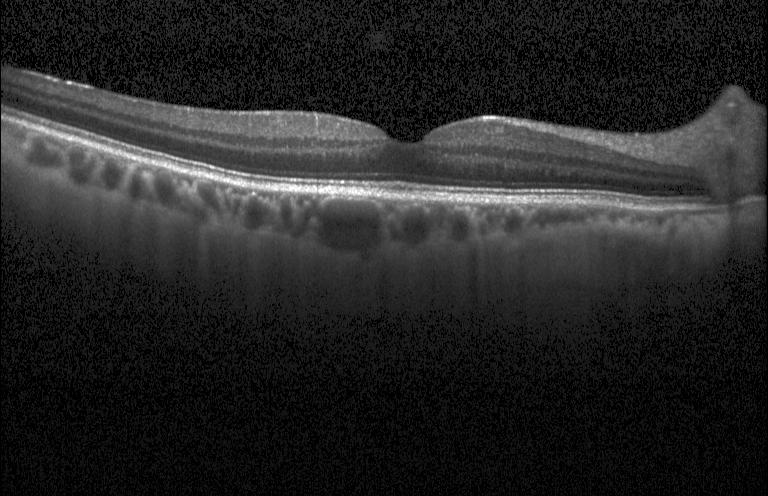 Neither choroidal neovascularization, diabetic macular edema, nor drusen.